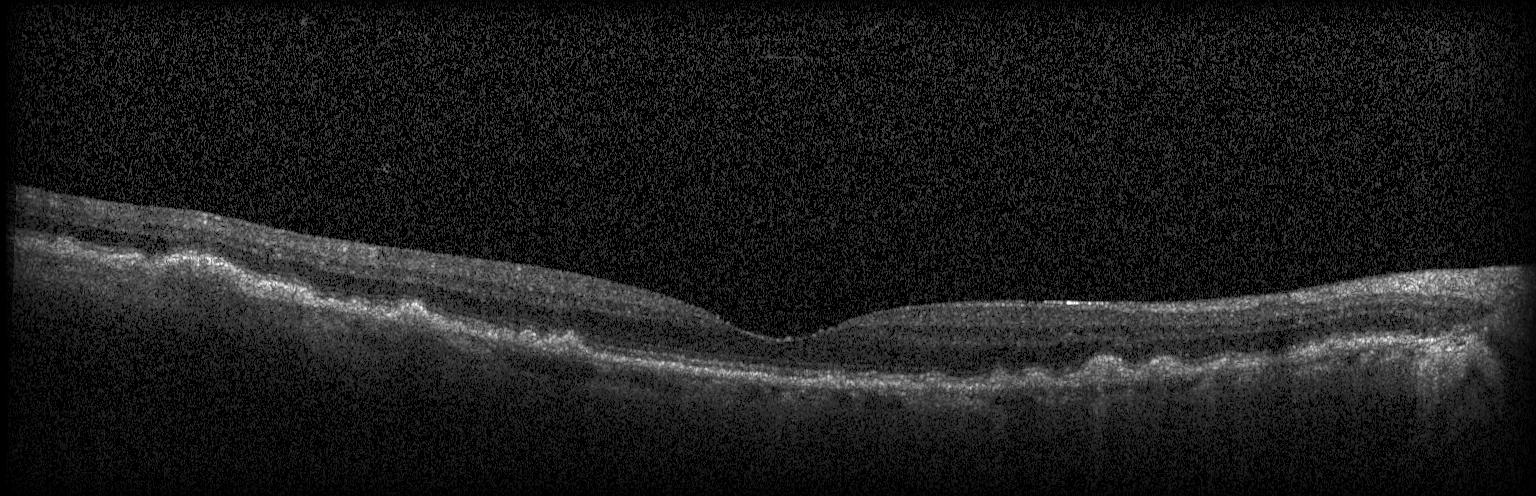 The scan shows sub-RPE drusenoid deposits.